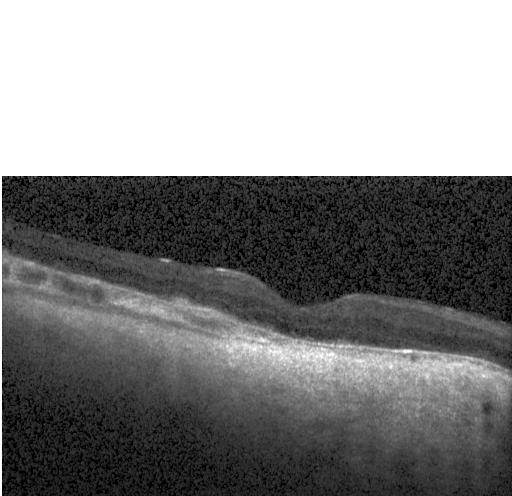

OCT scan showing CNV.